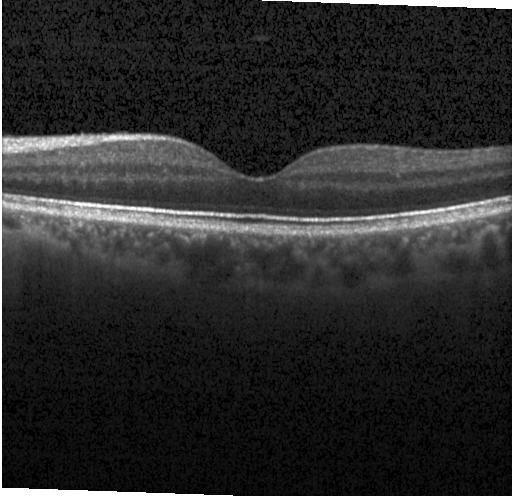
Optical coherence tomography B-scan
Diagnosis: neither choroidal neovascularization, diabetic macular edema, nor drusen.